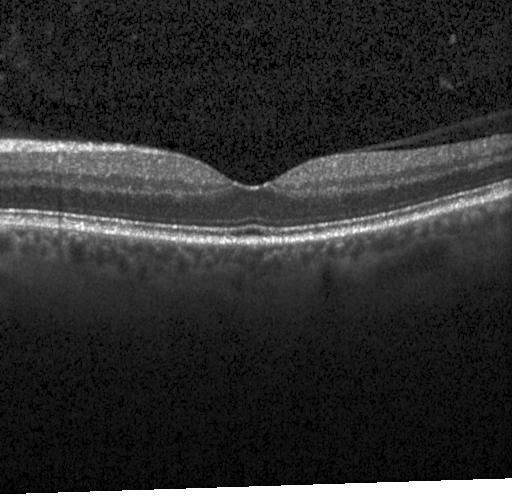
Finding: no CNV, DME, or drusen.